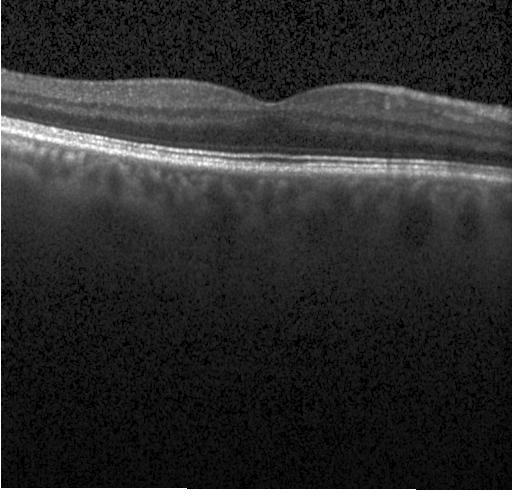 Diagnosis: no CNV, no DME, and no drusen.